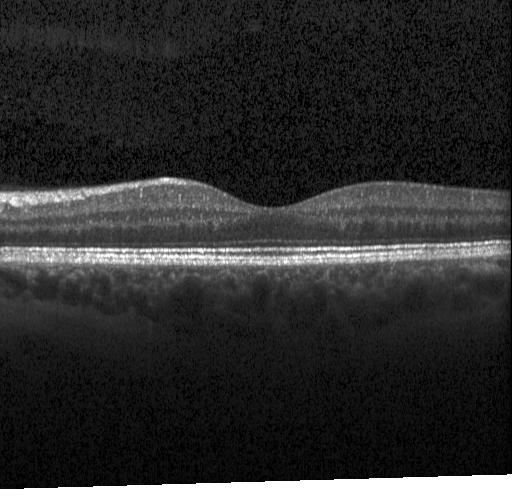 OCT line scan
The scan shows neither choroidal neovascularization, diabetic macular edema, nor drusen.